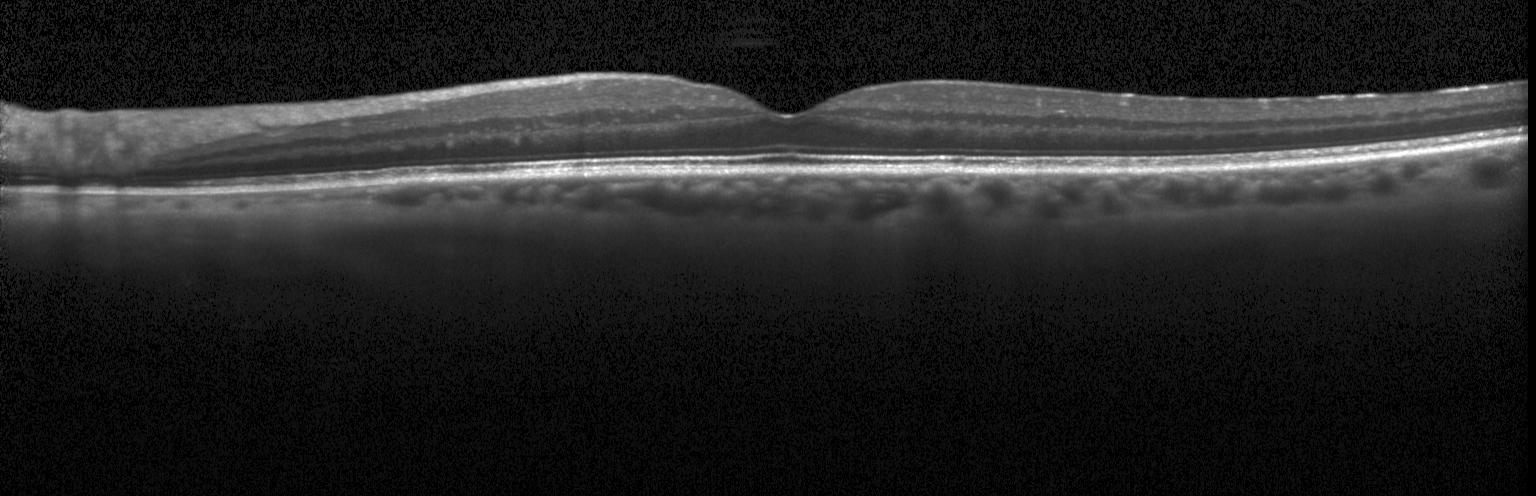
Finding: no evidence of CNV, DME, or drusen.